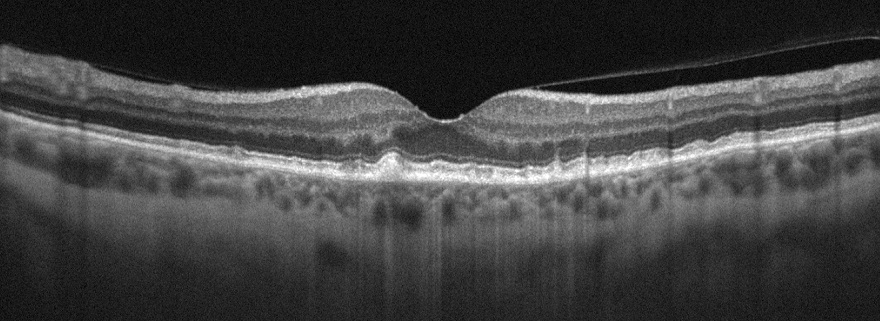
Diagnosis: age-related macular degeneration (AMD).